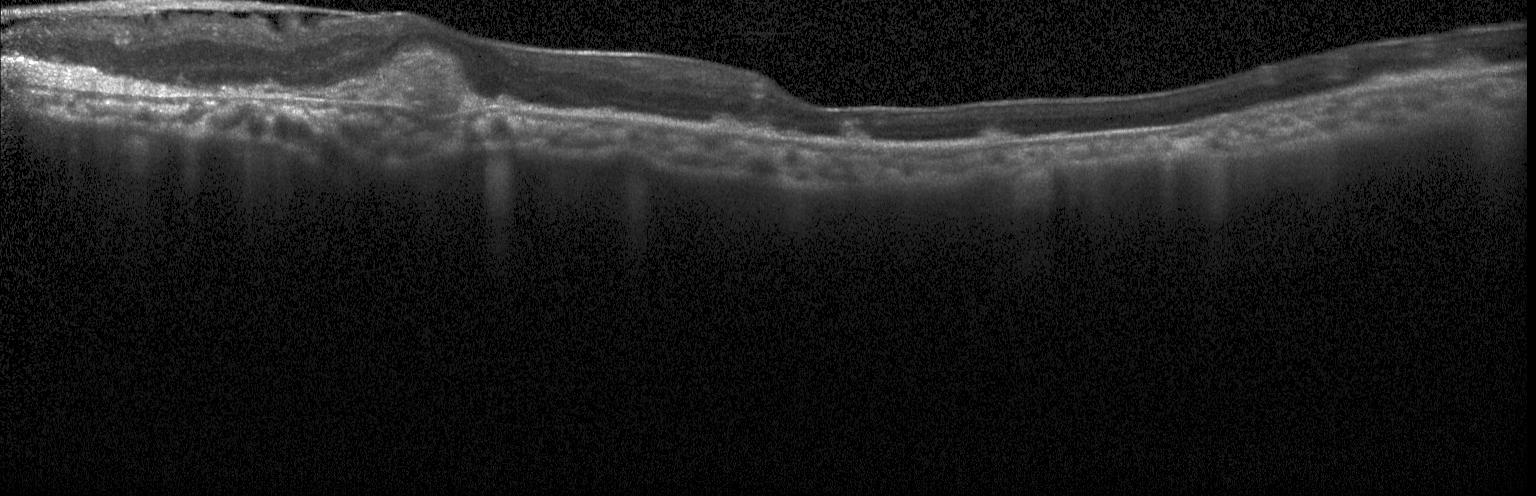
Retinal OCT B-scan, centered on the fovea
Finding: CNV.